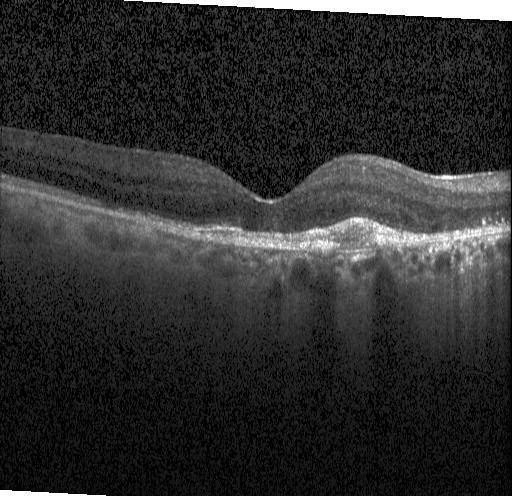 Optical coherence tomography B-scan. Acquired on a Heidelberg Spectralis. Centered on the fovea
Diagnosis: choroidal neovascularization (CNV).